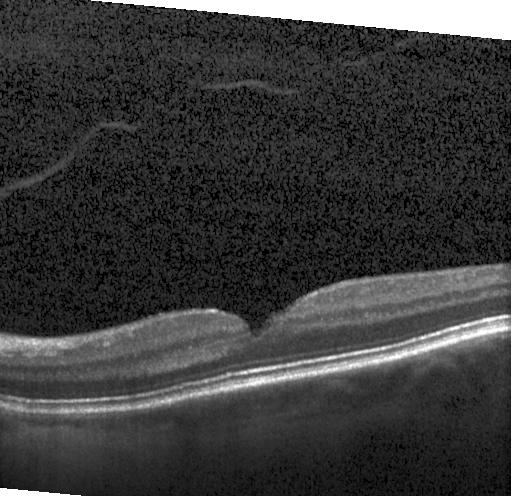 Fovea-centered; spectral-domain optical coherence tomography; retinal OCT B-scan.
The scan shows no choroidal neovascularization, no diabetic macular edema, and no drusen.